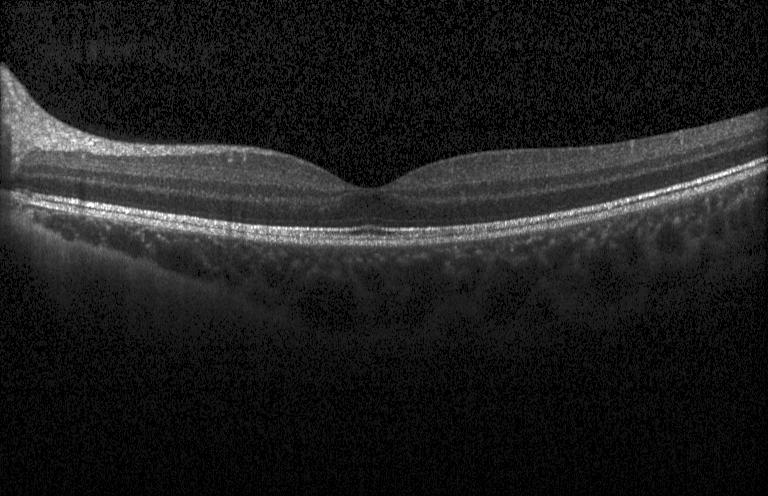
Macular OCT: neither choroidal neovascularization, diabetic macular edema, nor drusen.